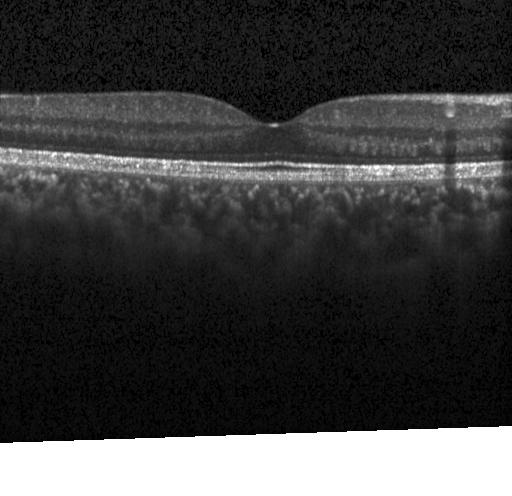 OCT B-scan. Through the macula.
Neither choroidal neovascularization, diabetic macular edema, nor drusen.